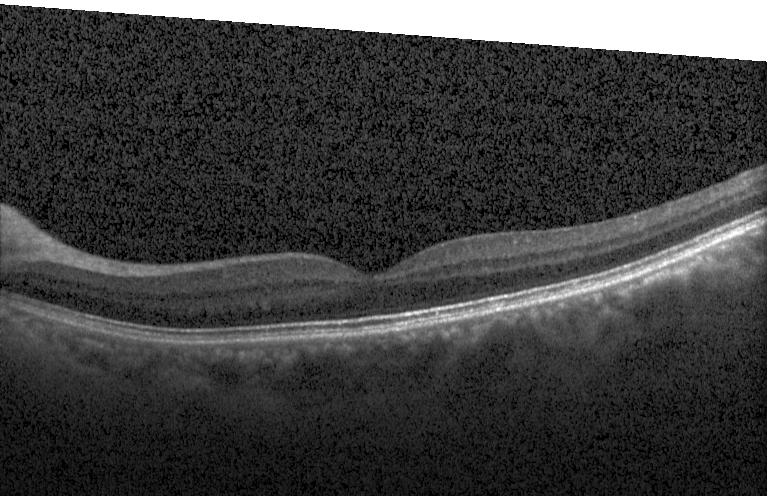
OCT scan showing no choroidal neovascularization, no diabetic macular edema, and no drusen.